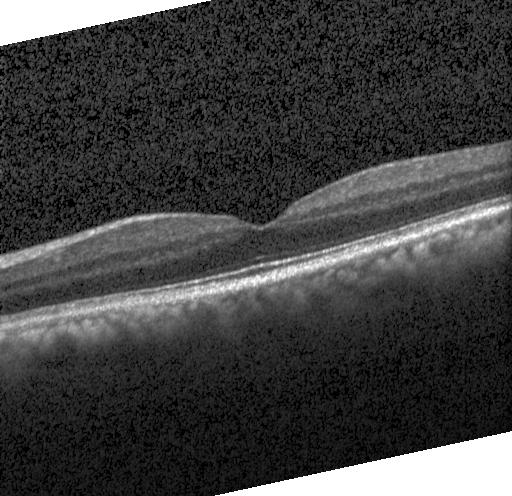
OCT line scan. Impression: no CNV, no DME, and no drusen.